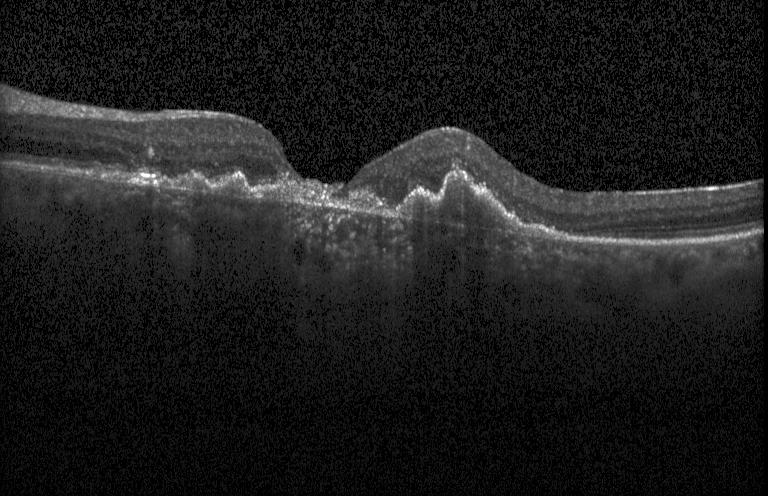
Spectral-domain OCT B-scan: CNV.